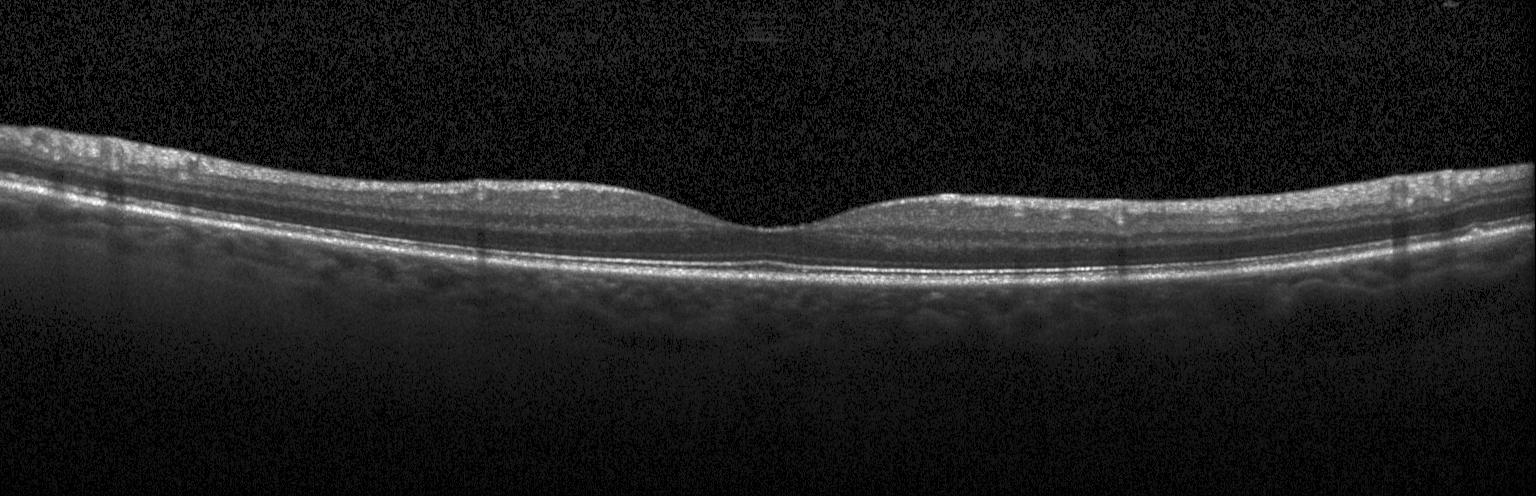 No CNV, no DME, and no drusen.